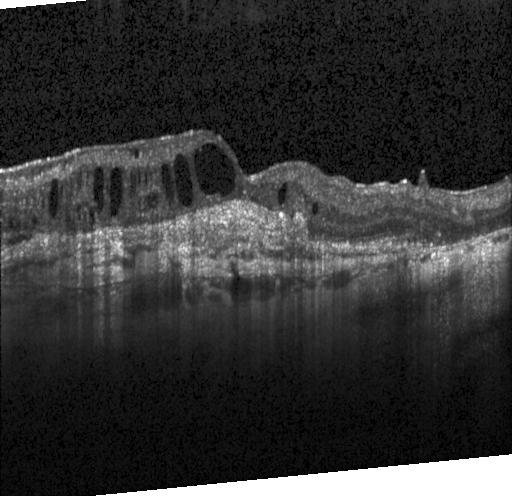

Horizontal scan through the fovea. OCT B-scan.
Assessment: a choroidal neovascular membrane.